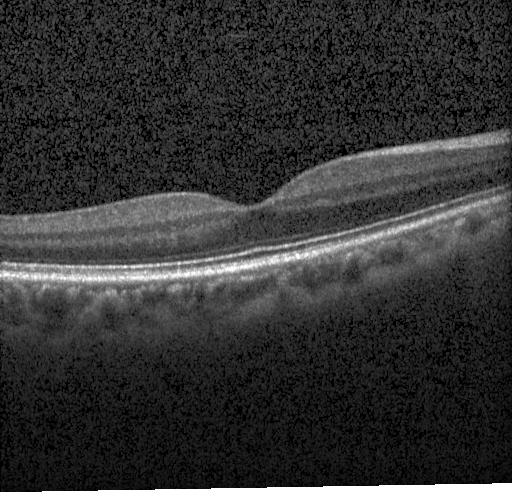 Diagnosis: no CNV, DME, or drusen.